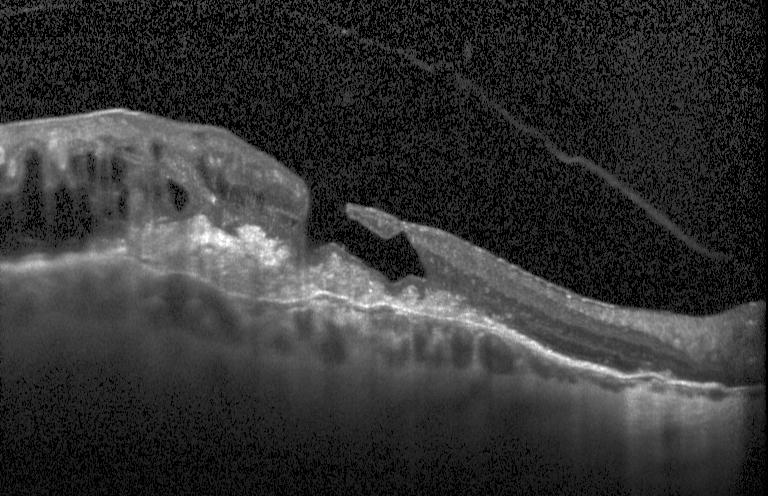 Macular OCT: a choroidal neovascular membrane.